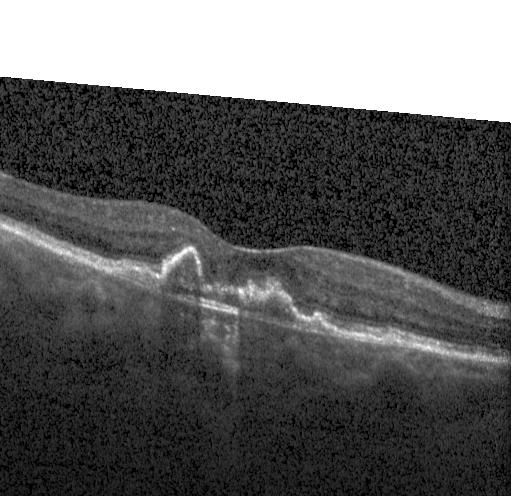 Optical coherence tomography scan. Fovea-centered. Spectral-domain OCT. Acquired on a Heidelberg Spectralis. Dx: choroidal neovascularization (CNV).